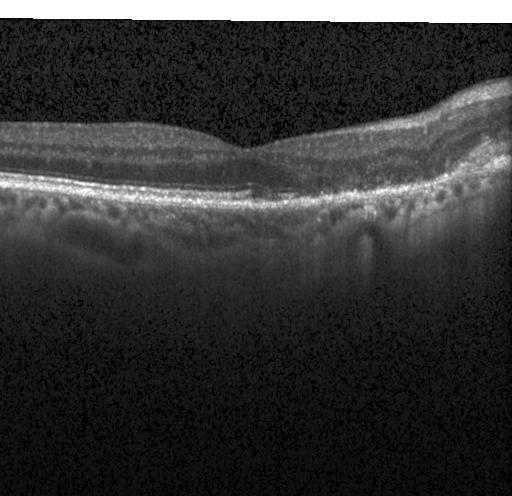

Impression: choroidal neovascularization.